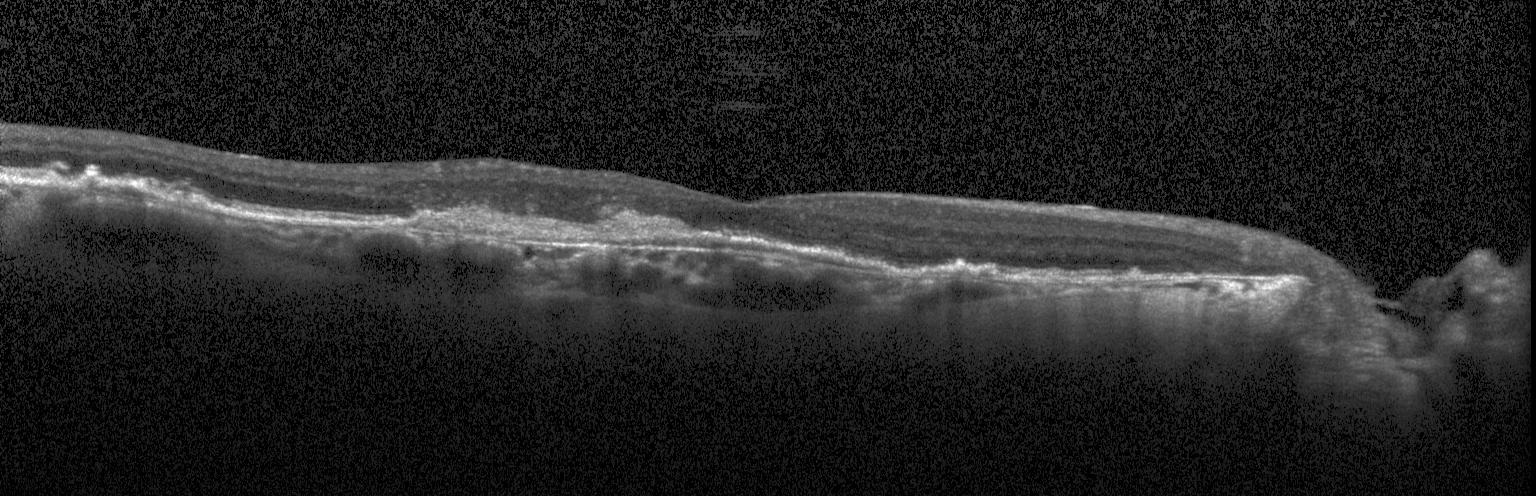
Diagnosis: a choroidal neovascular membrane.